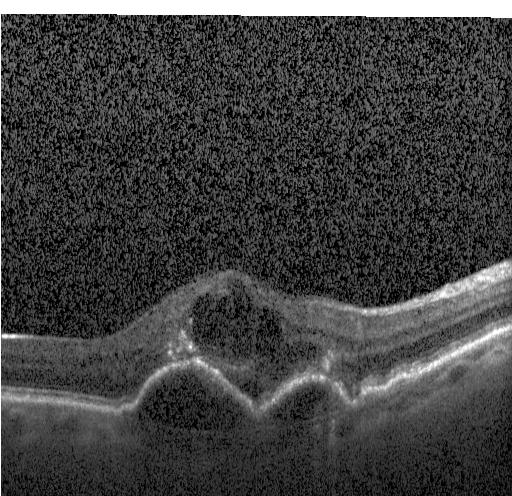
Retinal OCT B-scan · acquired on a Heidelberg Spectralis
OCT finding: CNV.